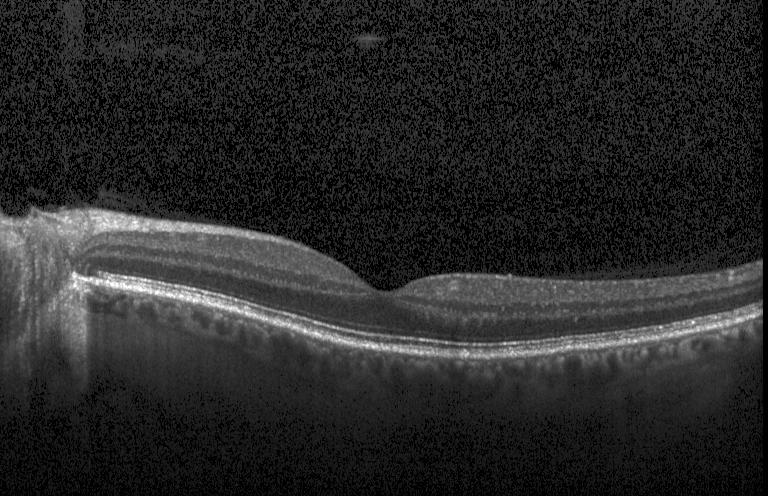

Spectral-domain OCT · horizontal scan through the fovea · retinal OCT cross-section. The scan shows neither choroidal neovascularization, diabetic macular edema, nor drusen.